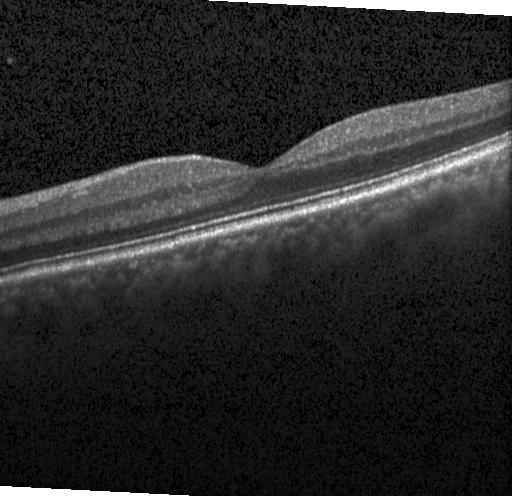 Heidelberg Spectralis OCT system. Retinal OCT cross-section. Spectral-domain optical coherence tomography. Through the macula — Impression: no choroidal neovascularization, diabetic macular edema, or drusen.